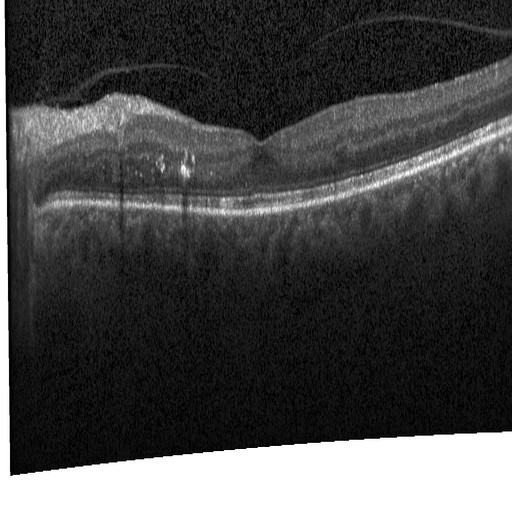
Optical coherence tomography B-scan. The scan shows DME.